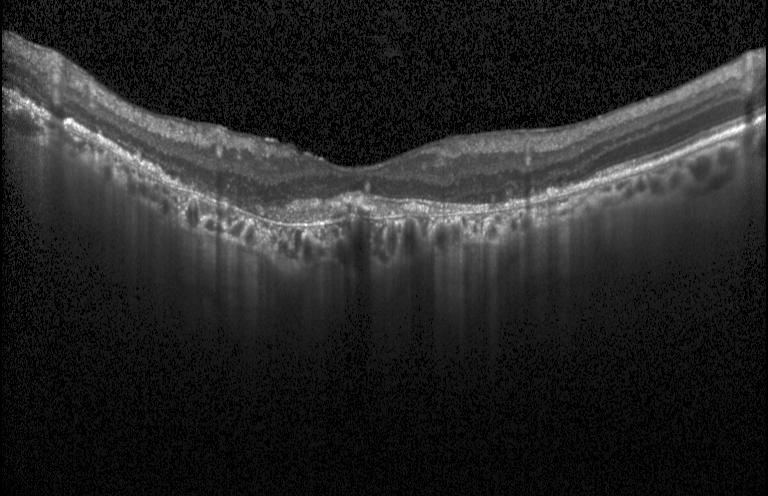

Optical coherence tomography B-scan
Finding: a choroidal neovascular membrane.